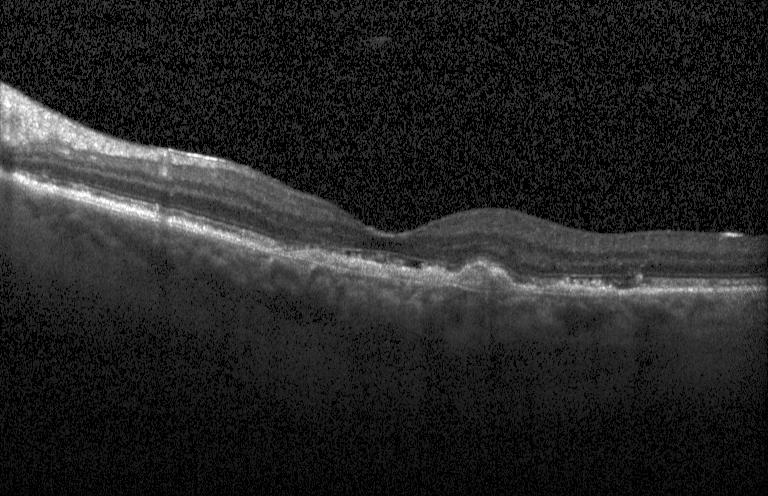 Retinal OCT B-scan. Finding: a choroidal neovascular membrane.